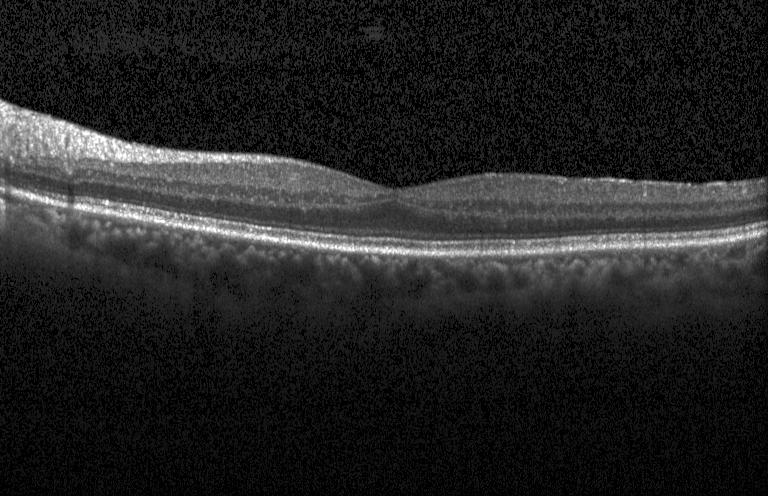

Spectral-domain OCT B-scan: no choroidal neovascularization, no diabetic macular edema, and no drusen.